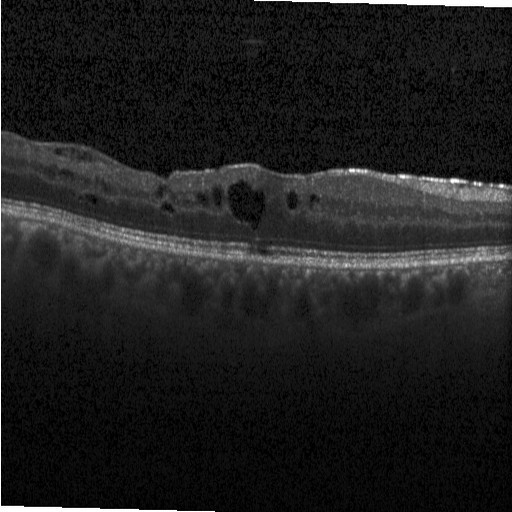 Optical coherence tomography B-scan — Diagnosis: diabetic macular edema (DME).